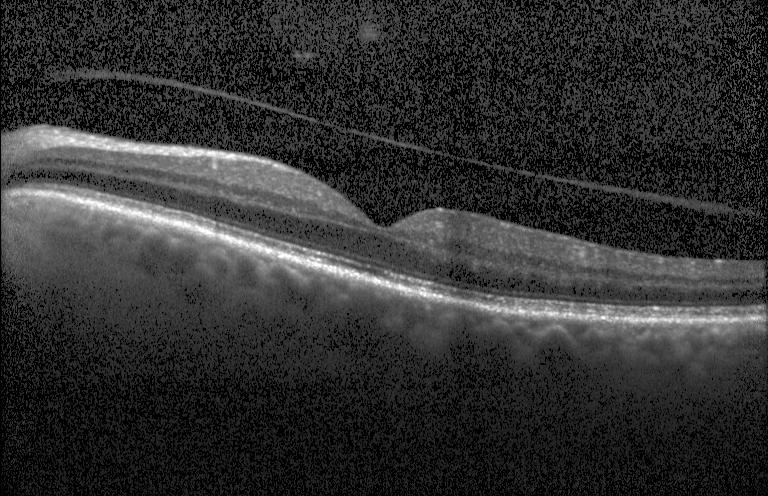
This B-scan demonstrates no choroidal neovascularization, diabetic macular edema, or drusen.